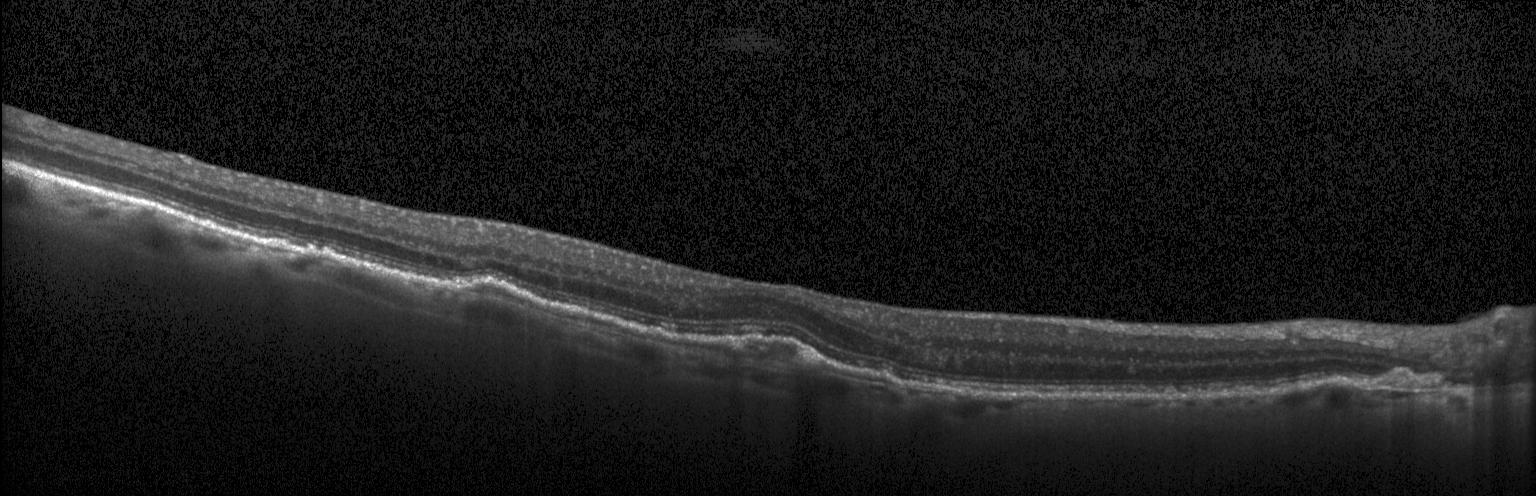

Diagnosis: CNV.